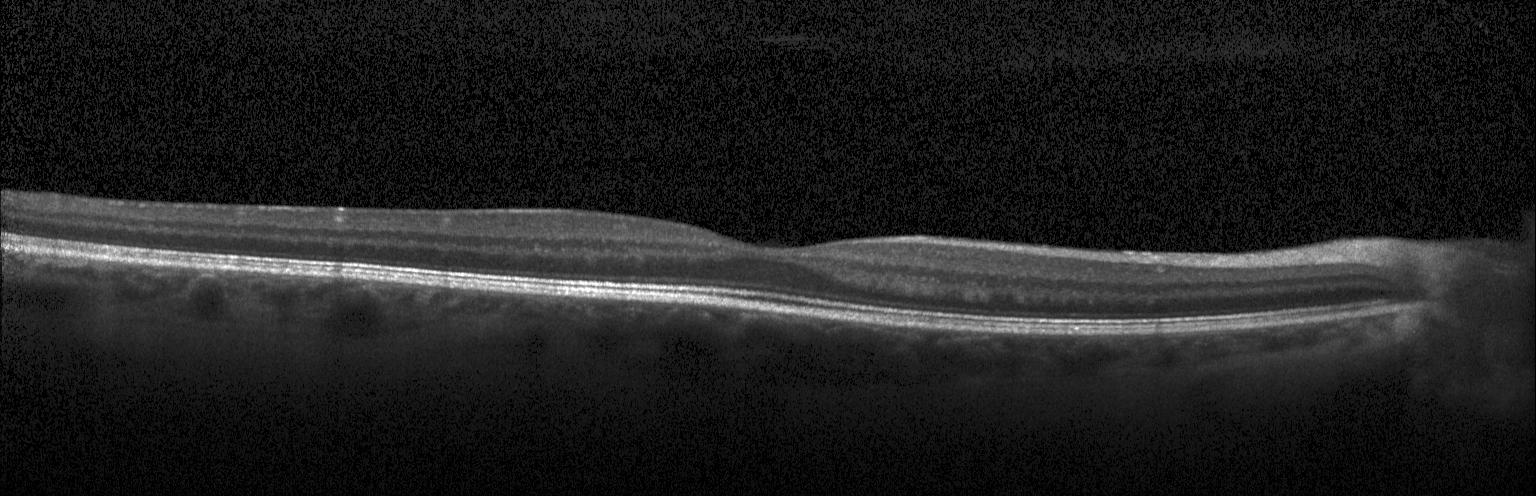 Diagnosis: no choroidal neovascularization, no diabetic macular edema, and no drusen.